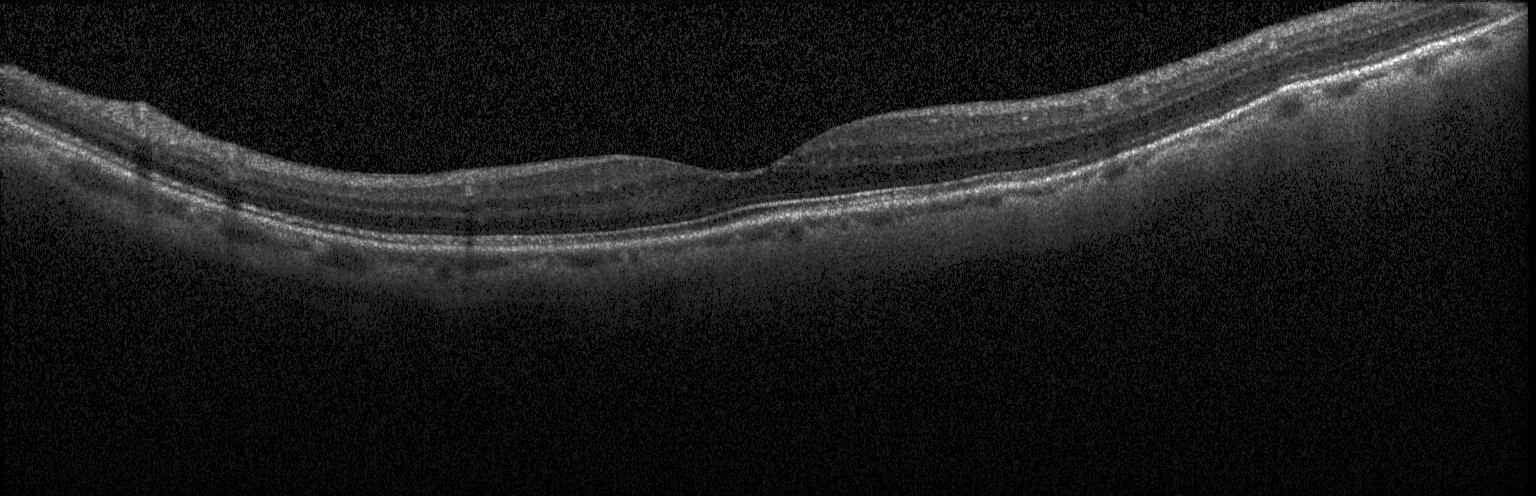
Retinal OCT cross-section showing no CNV, no DME, and no drusen.